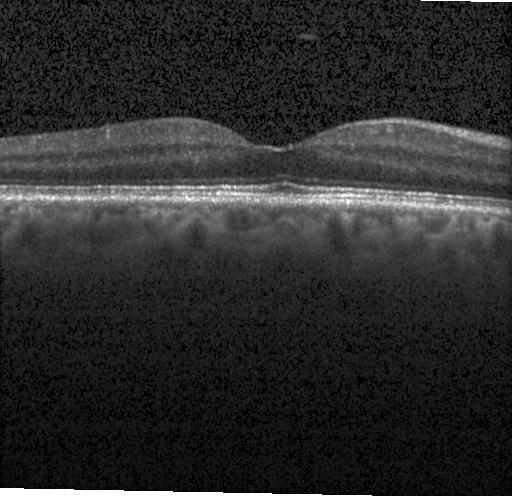 Fovea-centered; SD-OCT; retinal OCT B-scan.
Diagnosis: no CNV, no DME, and no drusen.